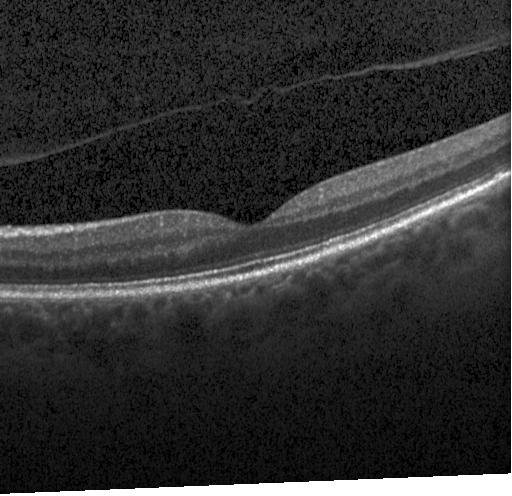
Spectral-domain OCT · retinal OCT B-scan.
Macular OCT: no choroidal neovascularization, no diabetic macular edema, and no drusen.